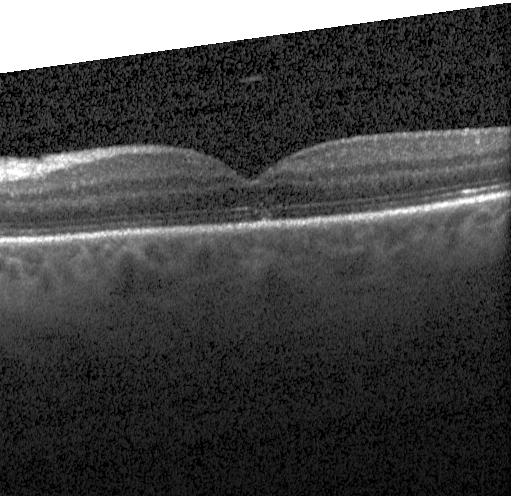 Optical coherence tomography scan.
Macular OCT: no CNV, no DME, and no drusen.